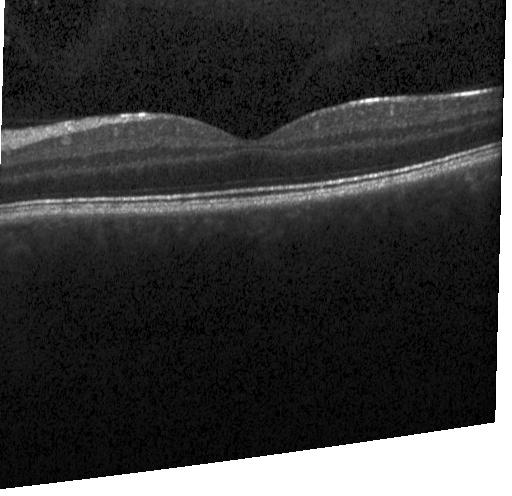 No choroidal neovascularization, diabetic macular edema, or drusen.